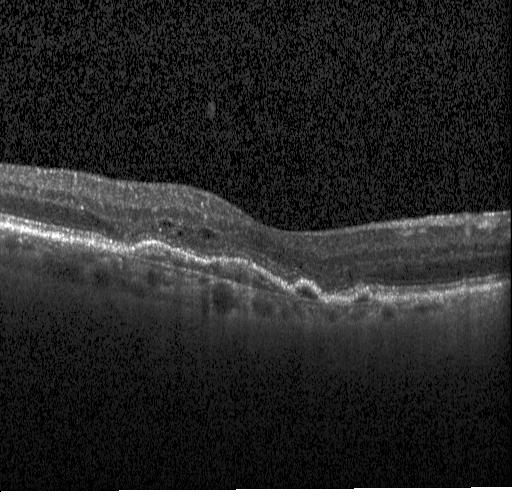 Retinal OCT cross-section. Macular scan. Instrument: Heidelberg Spectralis.
This B-scan demonstrates a choroidal neovascular membrane.